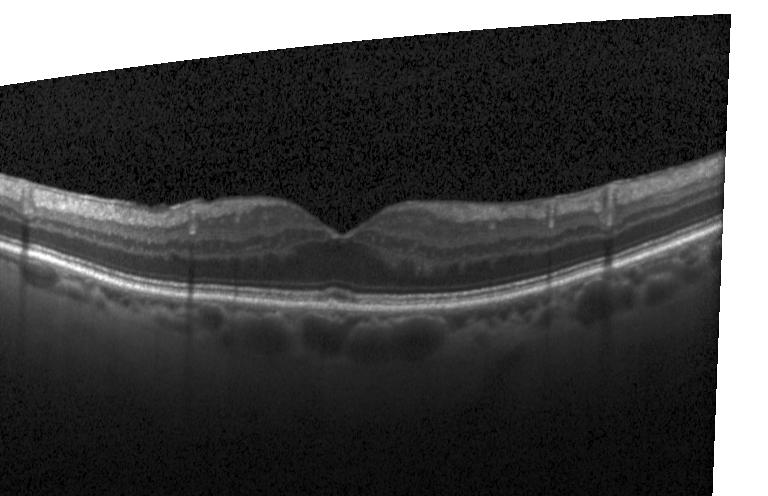 Fovea-centered. OCT B-scan. Spectral-domain optical coherence tomography. Heidelberg Spectralis OCT system. The scan shows neither choroidal neovascularization, diabetic macular edema, nor drusen.